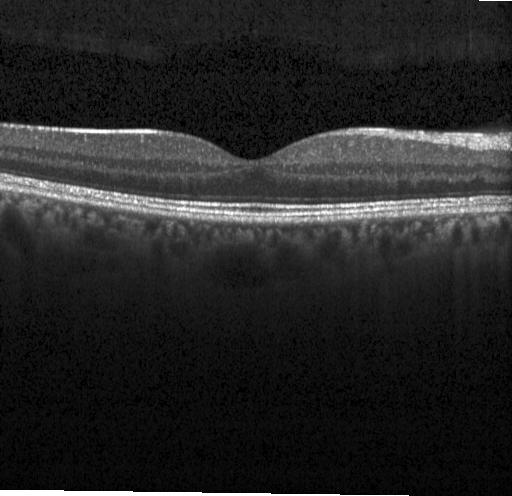
Optical coherence tomography B-scan.
The scan shows no CNV, no DME, and no drusen.